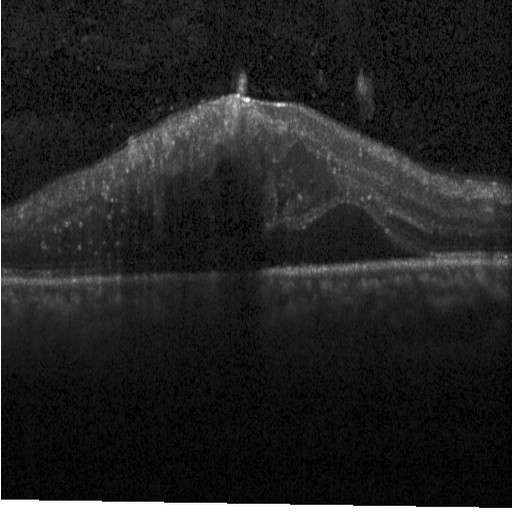 Diagnosis: diabetic macular edema (DME).